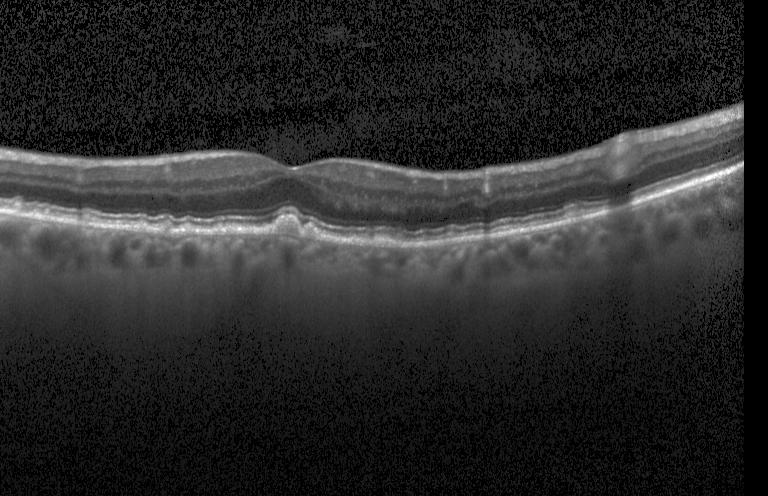

Diagnosis: sub-RPE drusenoid deposits.